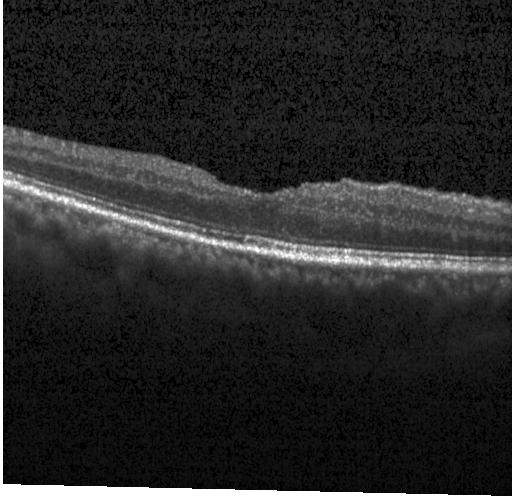

Acquired on a Heidelberg Spectralis, retinal OCT B-scan — No choroidal neovascularization, no diabetic macular edema, and no drusen.